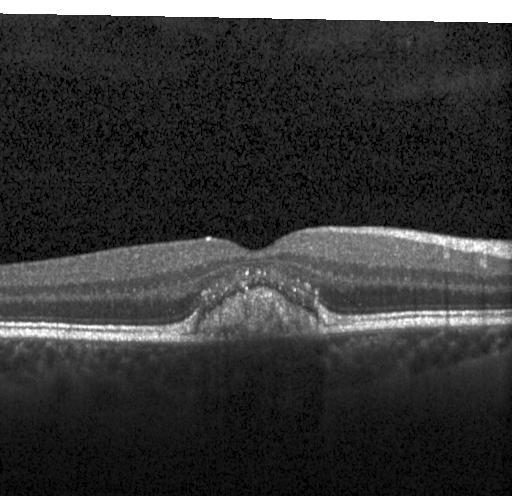

Optical coherence tomography scan — The scan shows a choroidal neovascular membrane.